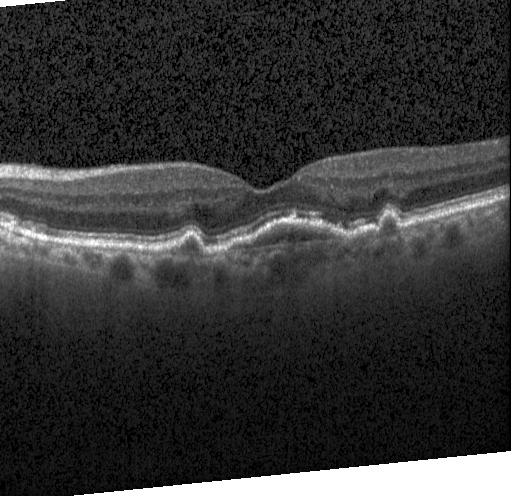 This B-scan demonstrates a choroidal neovascular membrane.